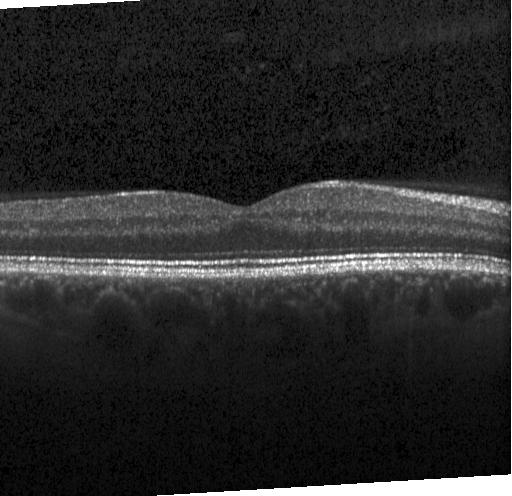
Optical coherence tomography scan.
Impression: no choroidal neovascularization, no diabetic macular edema, and no drusen.